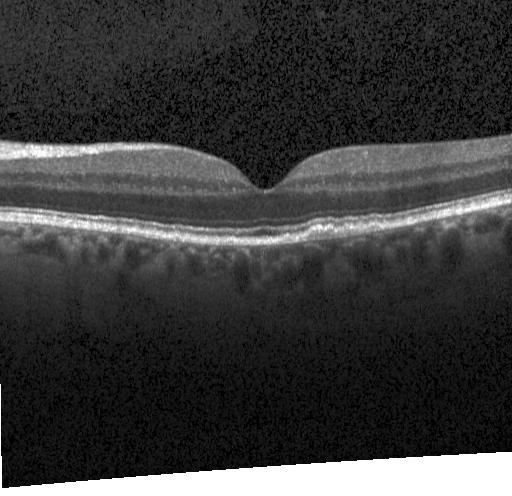

Finding: drusen.